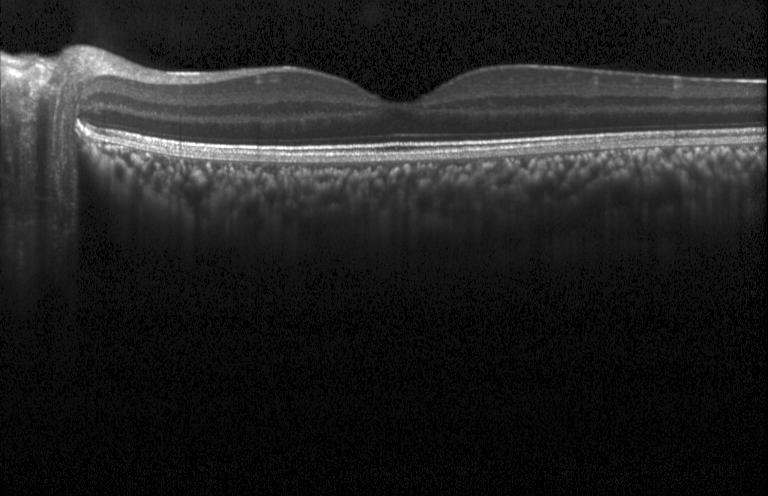

OCT B-scan.
Macular OCT: neither choroidal neovascularization, diabetic macular edema, nor drusen.